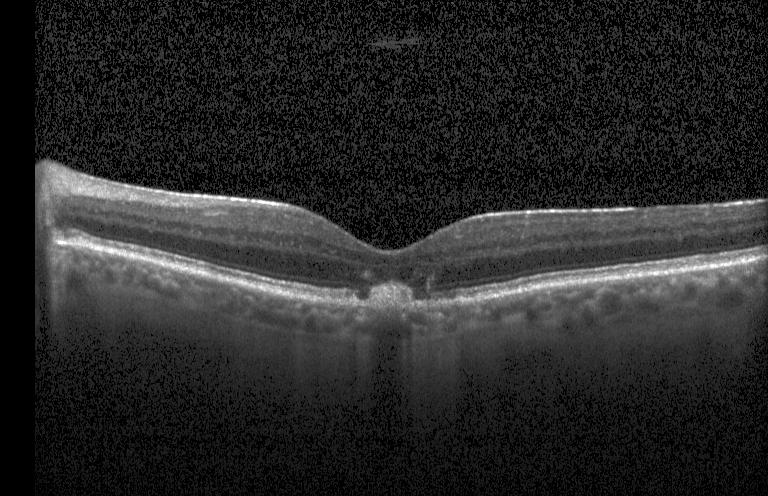

Impression: choroidal neovascularization (CNV).